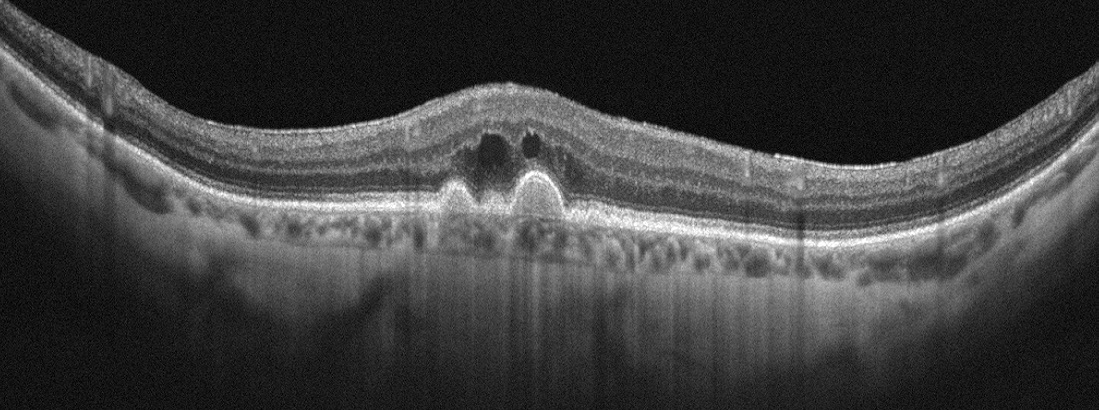
Optical coherence tomography B-scan. Acquired on an Optovue Avanti RTVue XR. Fovea-centered — This B-scan demonstrates age-related macular degeneration (AMD).